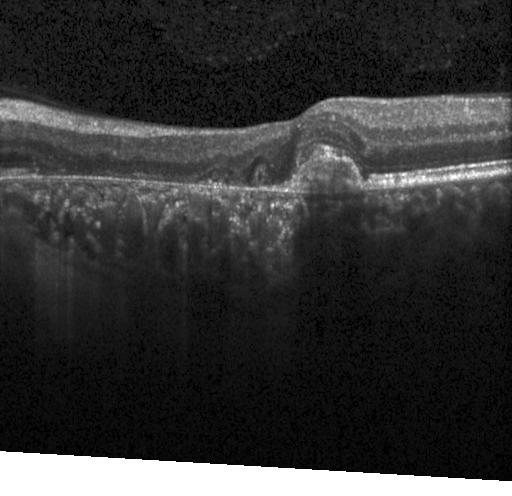
The scan shows a choroidal neovascular membrane.